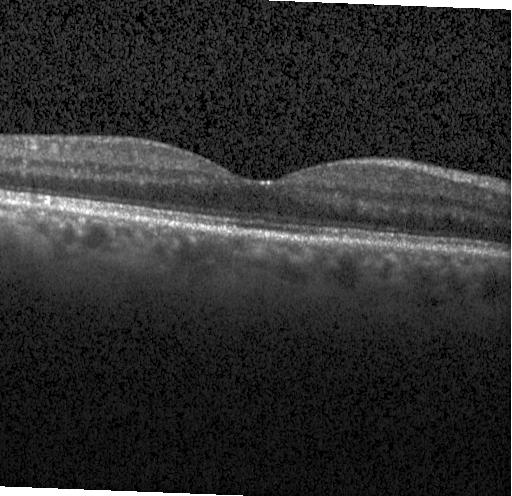 Heidelberg Spectralis, spectral-domain optical coherence tomography, retinal OCT B-scan — Diagnosis: no evidence of choroidal neovascularization, diabetic macular edema, or drusen.